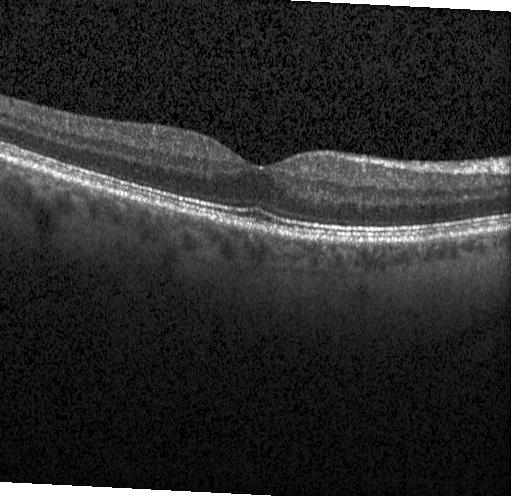 Diagnosis: no choroidal neovascularization, diabetic macular edema, or drusen.